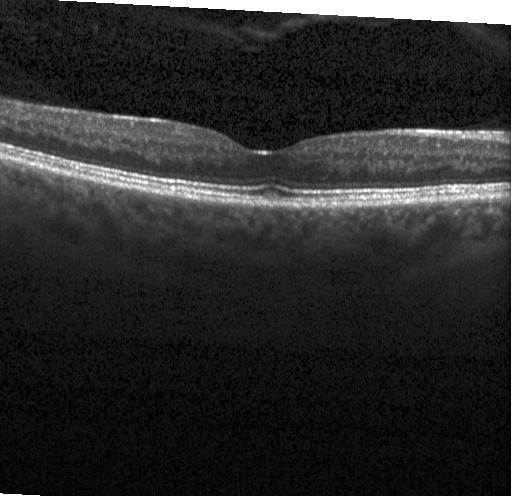 Heidelberg Spectralis OCT system · macular scan · optical coherence tomography B-scan — Diagnosis: no choroidal neovascularization, diabetic macular edema, or drusen.